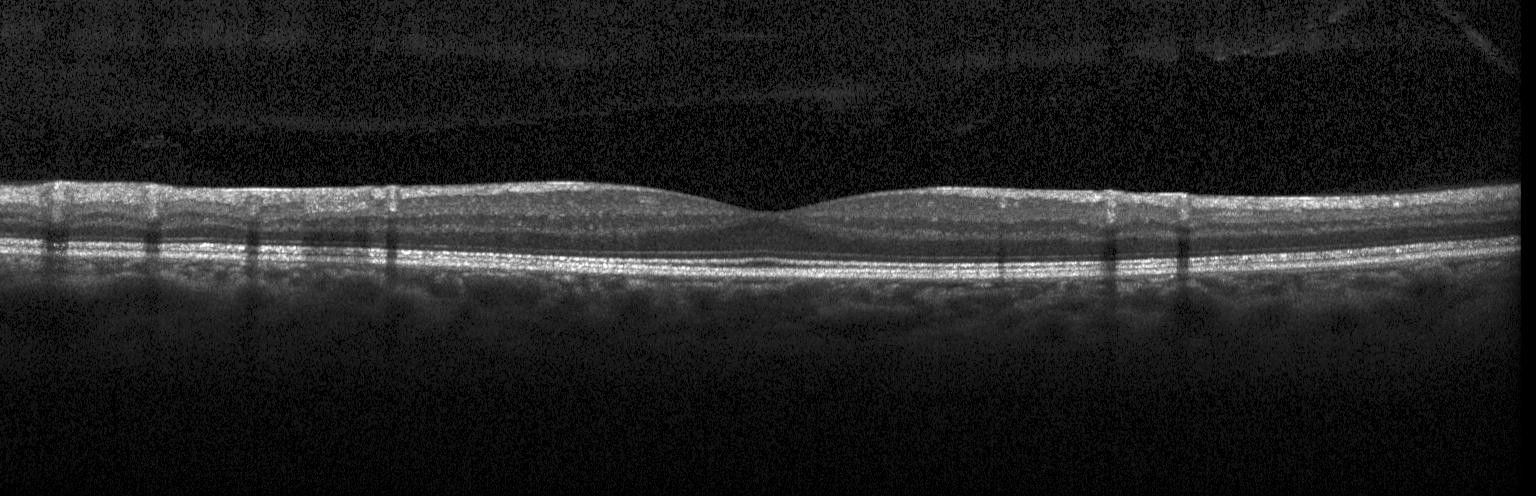 OCT B-scan · SD-OCT.
Impression: no evidence of CNV, DME, or drusen.